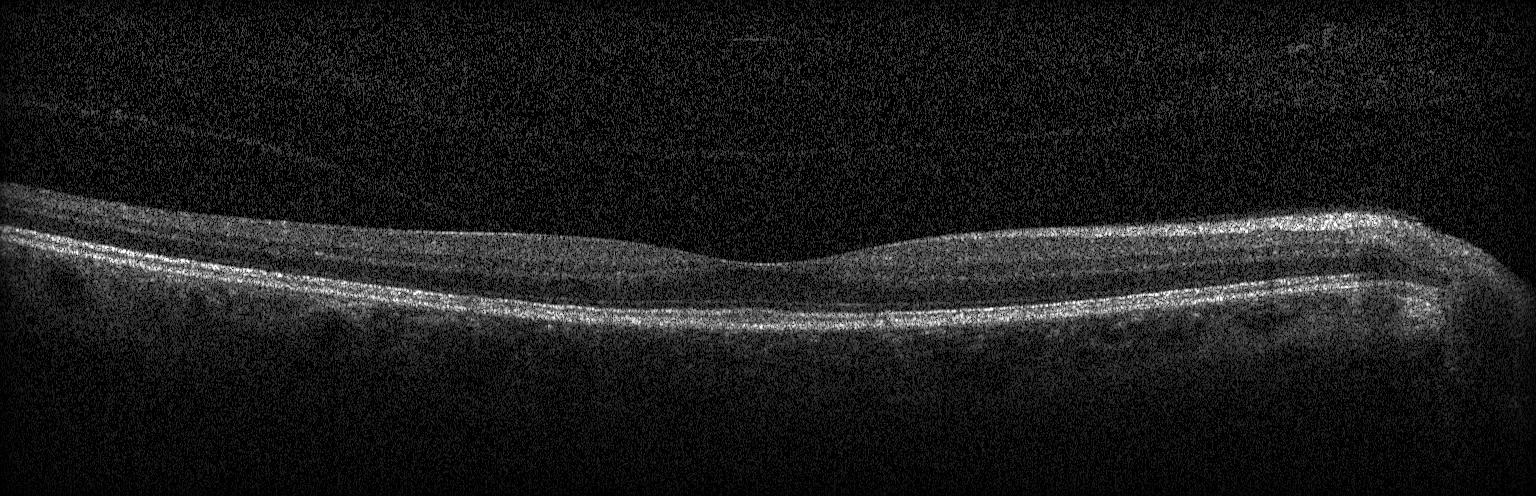
Optical coherence tomography scan · SD-OCT · horizontal scan through the fovea · Heidelberg Spectralis — Impression: no evidence of choroidal neovascularization, diabetic macular edema, or drusen.